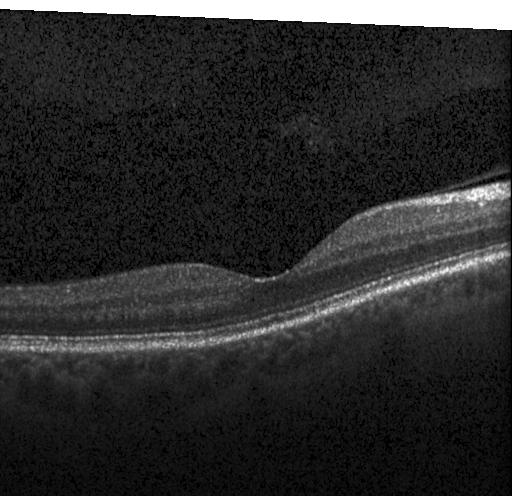

Diagnosis: no evidence of choroidal neovascularization, diabetic macular edema, or drusen.